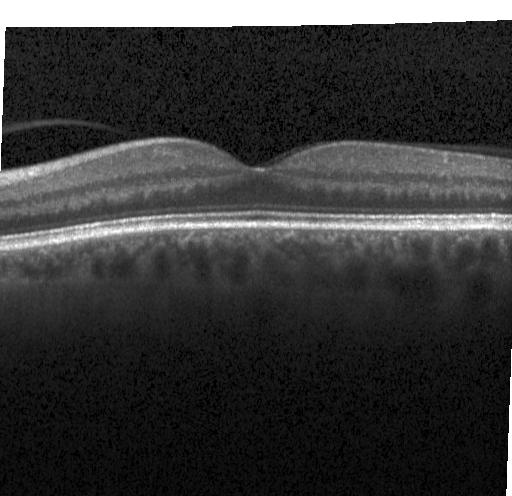
Finding: no choroidal neovascularization, diabetic macular edema, or drusen.